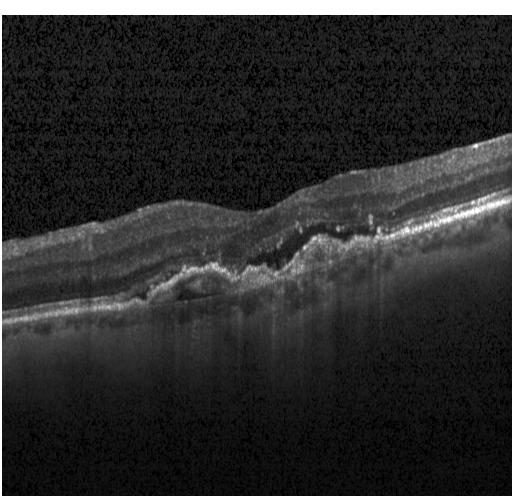
Optical coherence tomography scan.
Finding: choroidal neovascularization.